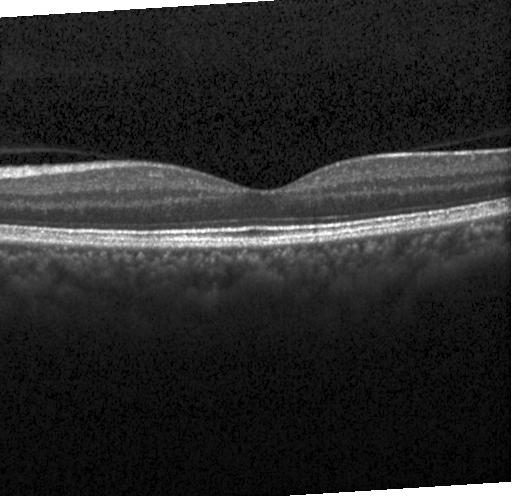
Assessment: no choroidal neovascularization, no diabetic macular edema, and no drusen.